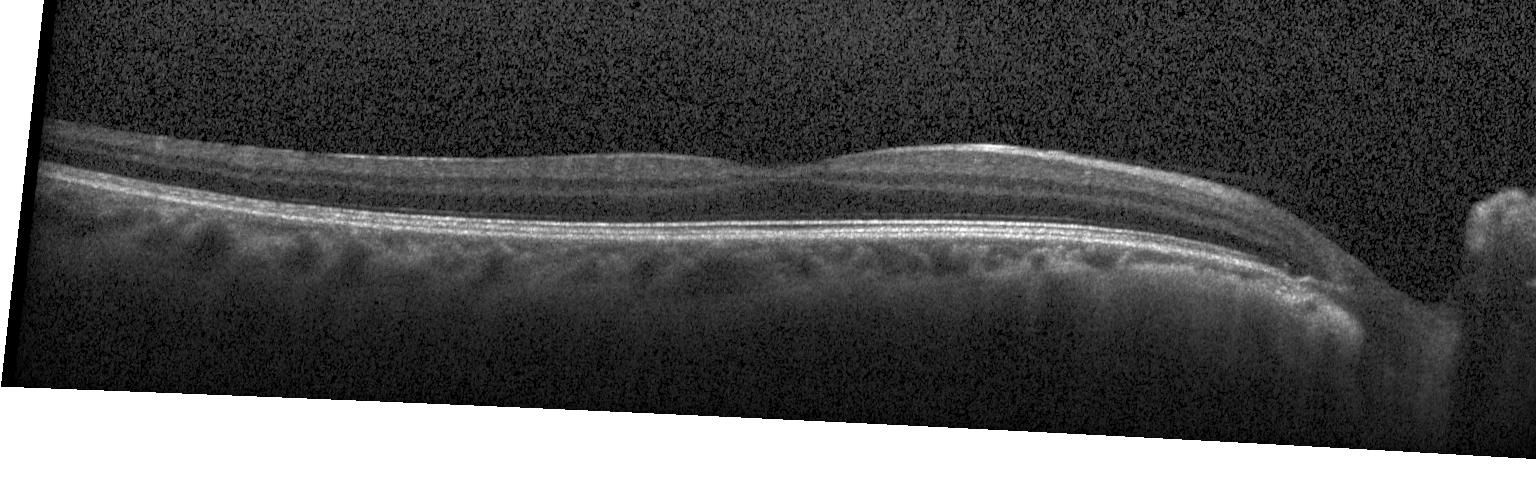 Impression: no CNV, DME, or drusen.